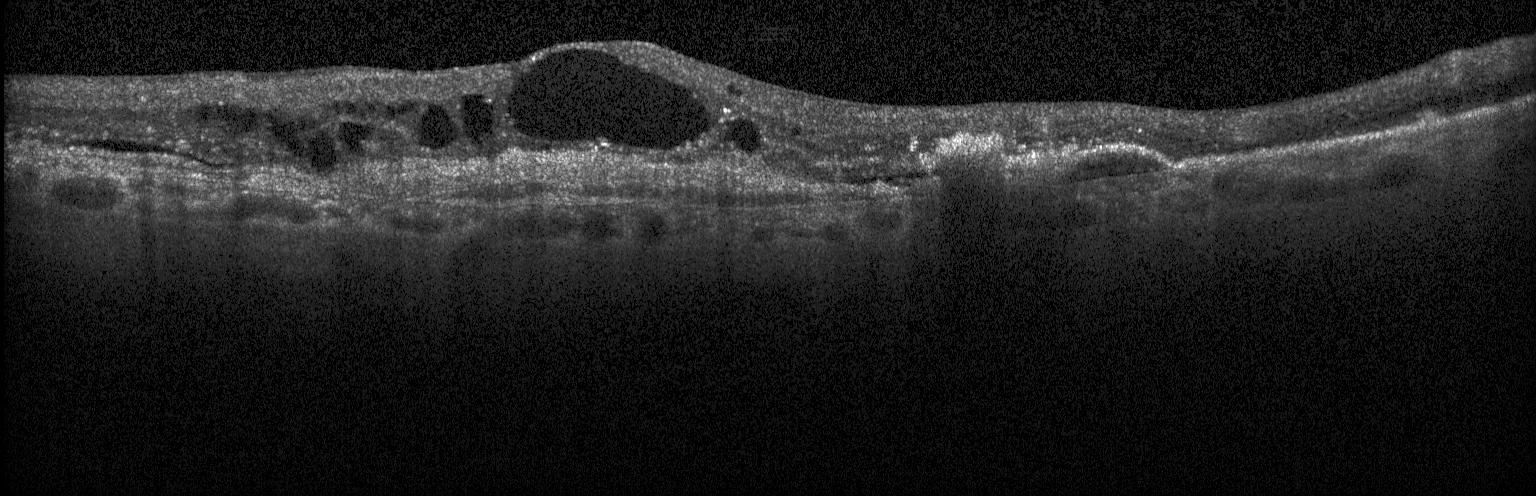

Macular OCT: choroidal neovascularization (CNV).